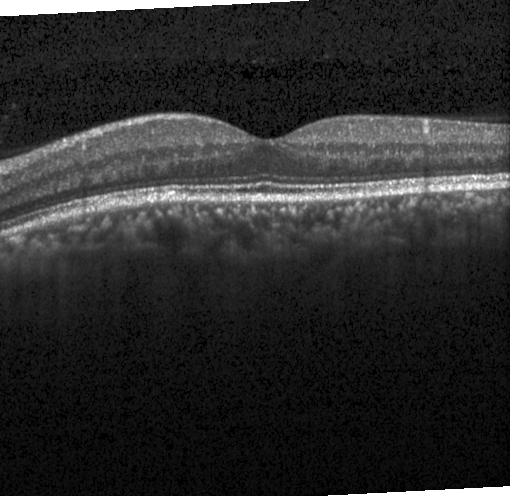
Spectral-domain optical coherence tomography · retinal OCT B-scan · centered on the fovea · Heidelberg Spectralis OCT system.
Impression: neither CNV, DME, nor drusen.